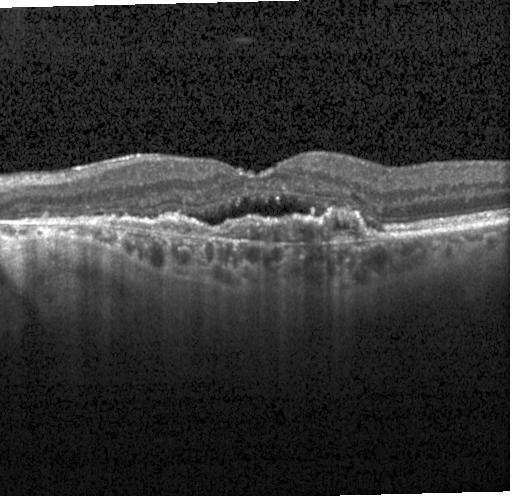
Instrument: Heidelberg Spectralis, OCT line scan. The scan shows CNV.